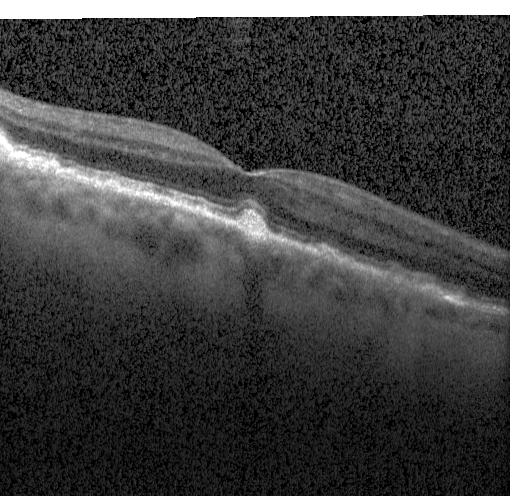
Through the macula. SD-OCT. Retinal OCT B-scan — Diagnosis: drusen.